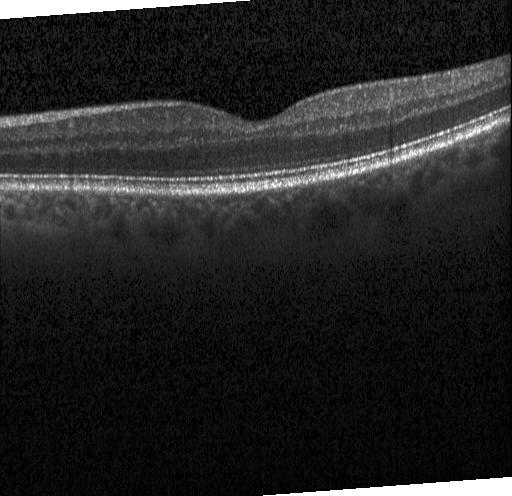

Spectral-domain OCT, macular scan, OCT B-scan, acquired on a Heidelberg Spectralis — Finding: no choroidal neovascularization, diabetic macular edema, or drusen.